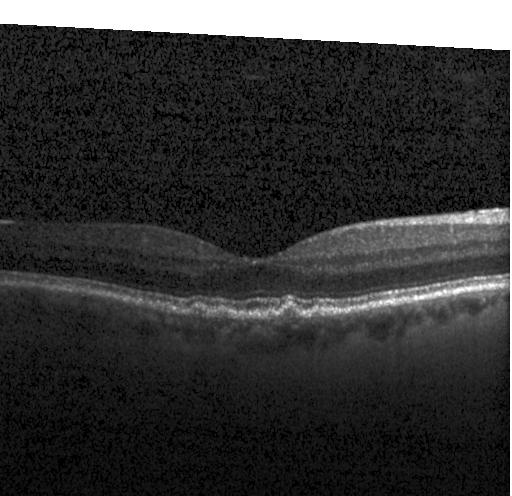 Diagnosis: drusen.